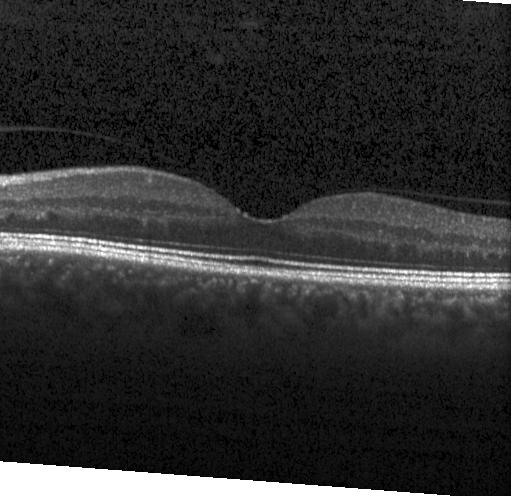 Macular OCT: no choroidal neovascularization, diabetic macular edema, or drusen.